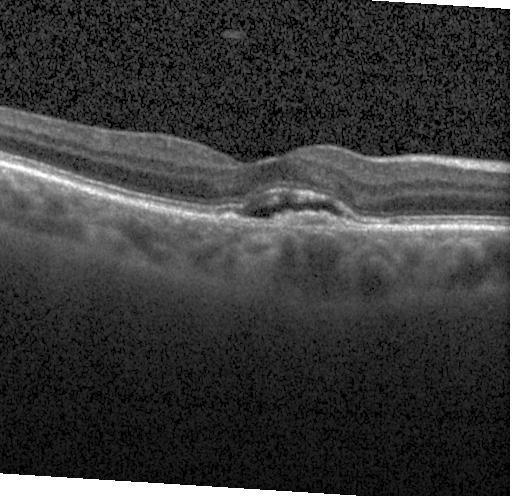
Instrument: Heidelberg Spectralis. Retinal OCT B-scan. Through the macula. Assessment: CNV.